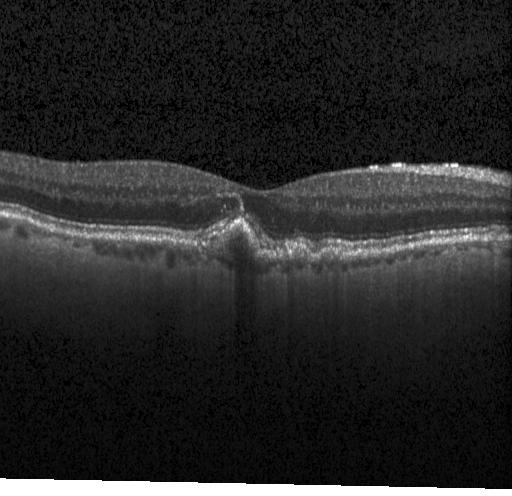
OCT B-scan
Diagnosis: drusen.